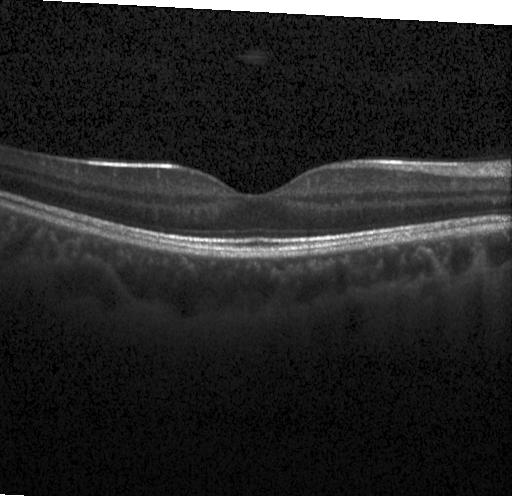 Acquired on a Heidelberg Spectralis · OCT line scan · spectral-domain OCT · centered on the fovea.
Diagnosis: no evidence of choroidal neovascularization, diabetic macular edema, or drusen.